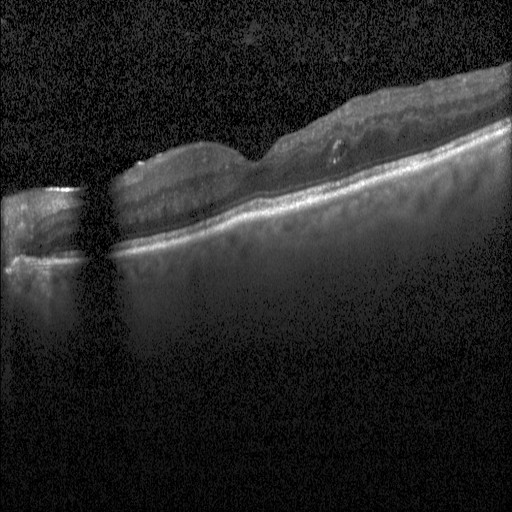
Heidelberg Spectralis. Retinal OCT cross-section. Macular scan. Spectral-domain optical coherence tomography.
Dx: DME.